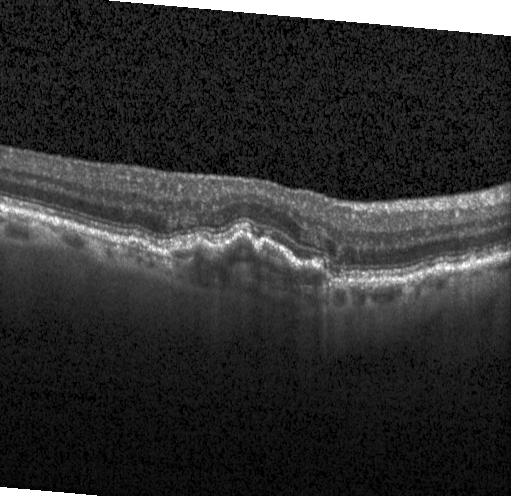

Instrument: Heidelberg Spectralis. Macular scan. Optical coherence tomography scan
A choroidal neovascular membrane.